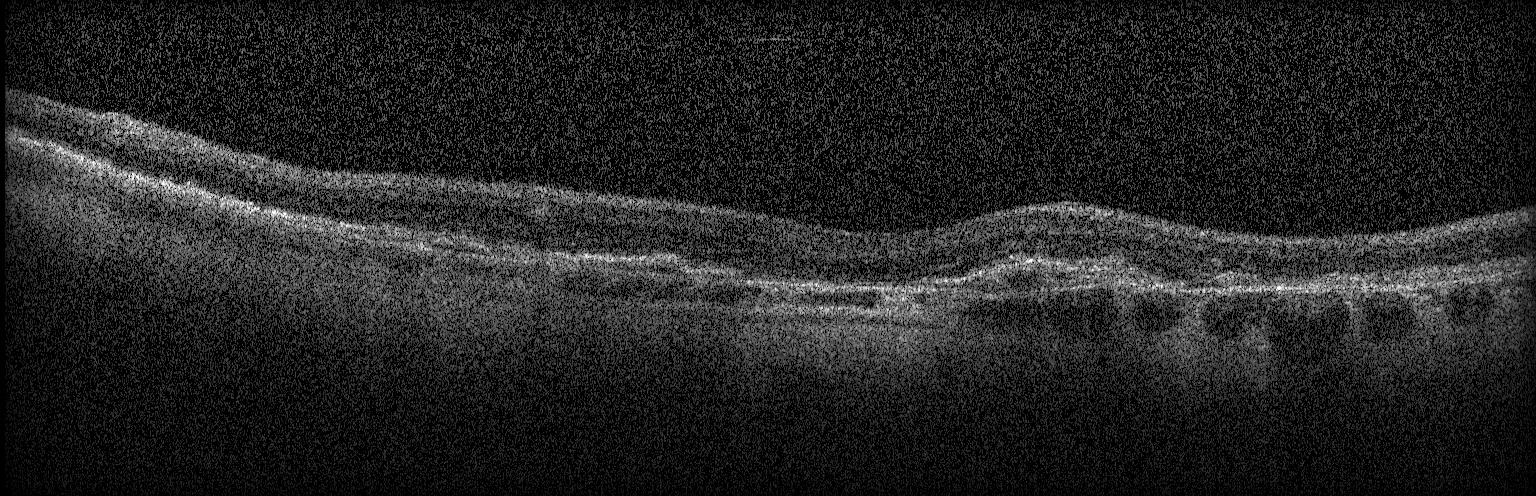
Spectral-domain OCT B-scan: a choroidal neovascular membrane.